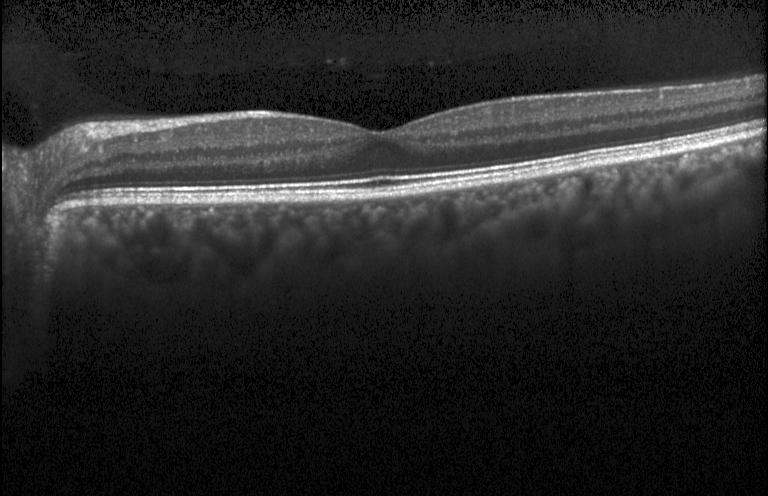 Macular OCT: no evidence of CNV, DME, or drusen.